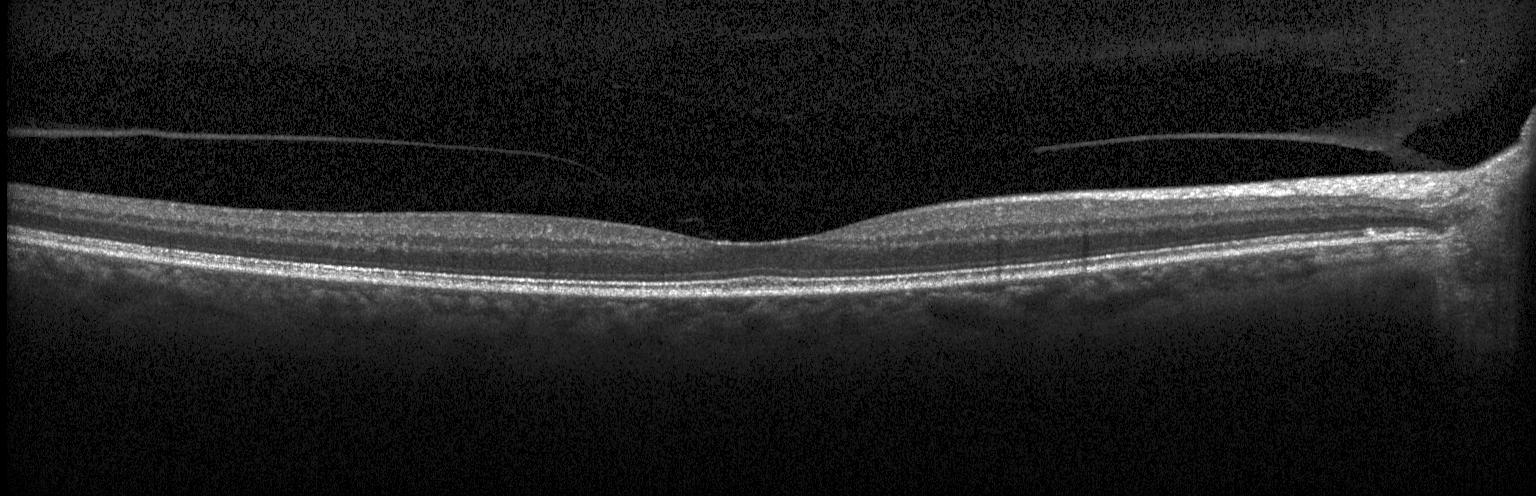

Retinal OCT cross-section showing no choroidal neovascularization, diabetic macular edema, or drusen.